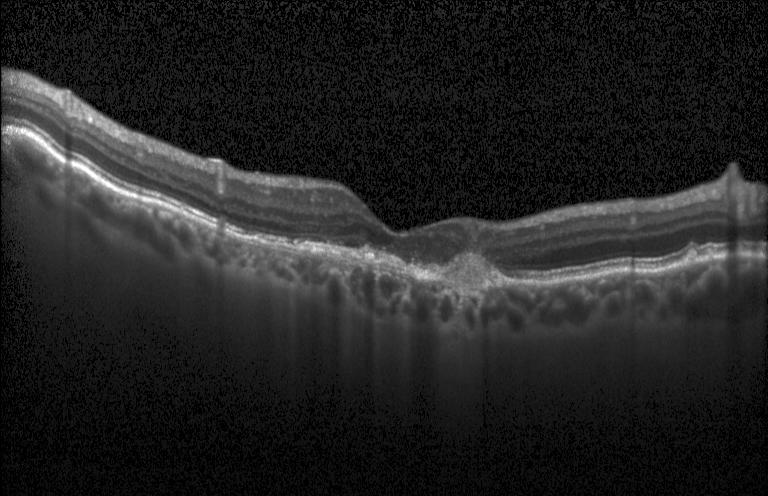 Retinal OCT cross-section. Spectral-domain OCT
This B-scan demonstrates a choroidal neovascular membrane.